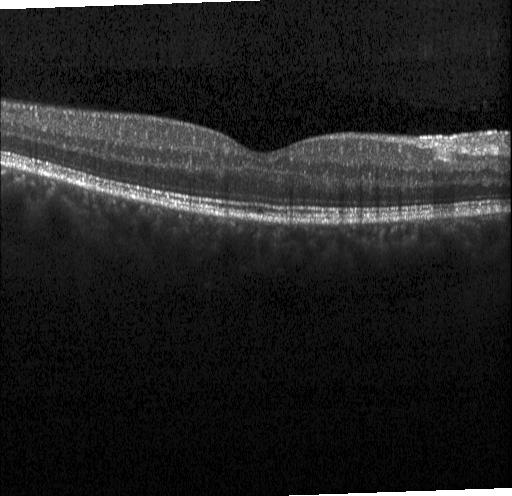

Retinal OCT B-scan, Heidelberg Spectralis.
Impression: neither choroidal neovascularization, diabetic macular edema, nor drusen.